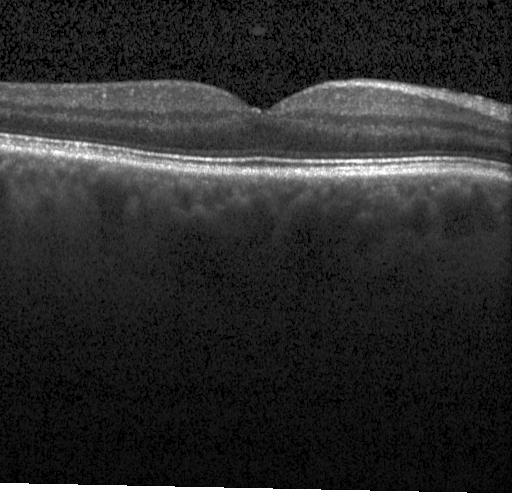

Optical coherence tomography B-scan.
Impression: neither CNV, DME, nor drusen.